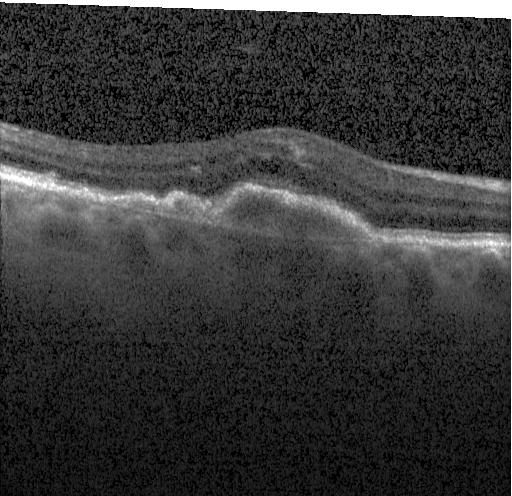
This B-scan demonstrates choroidal neovascularization (CNV).